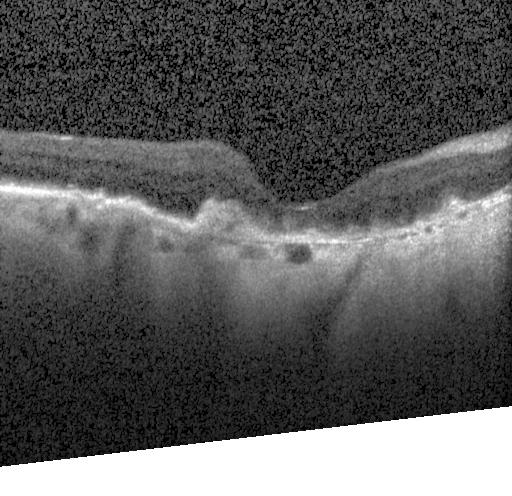
OCT scan showing choroidal neovascularization (CNV).